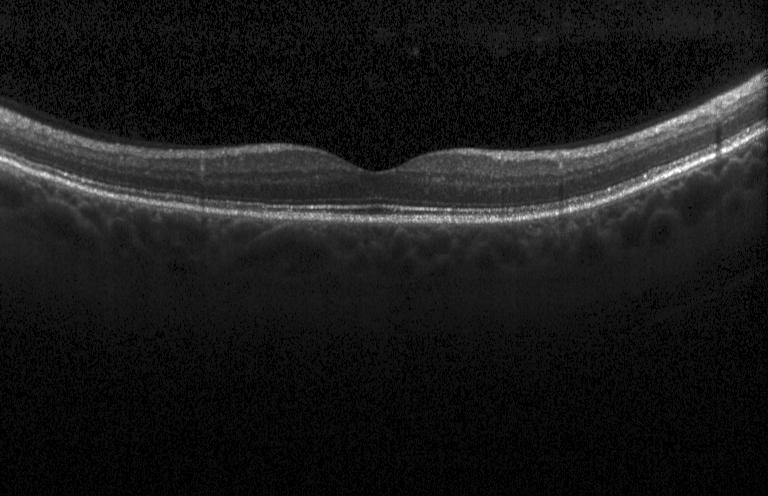
Optical coherence tomography B-scan. Assessment: neither choroidal neovascularization, diabetic macular edema, nor drusen.